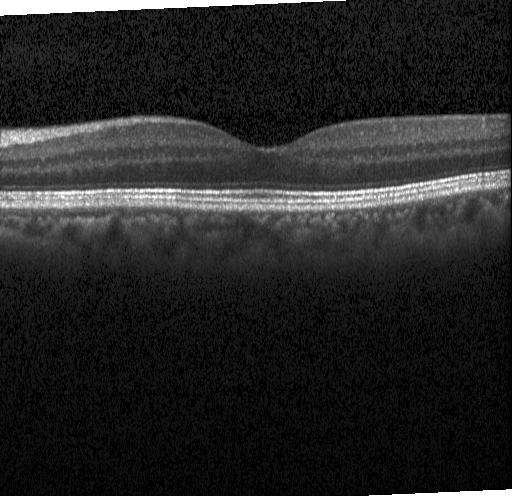
Spectral-domain optical coherence tomography · through the macula · retinal OCT B-scan. Macular OCT: neither choroidal neovascularization, diabetic macular edema, nor drusen.